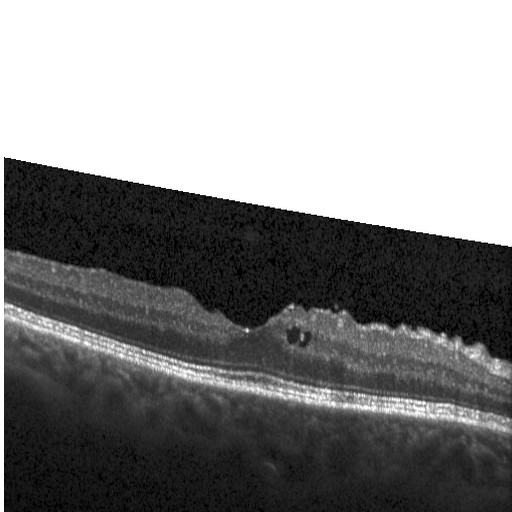
Spectral-domain OCT; Heidelberg Spectralis OCT system; optical coherence tomography B-scan; centered on the fovea — Assessment: diabetic macular edema.